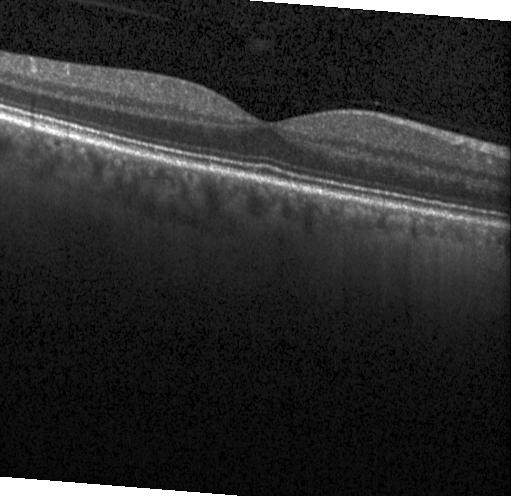
Diagnosis: neither choroidal neovascularization, diabetic macular edema, nor drusen.